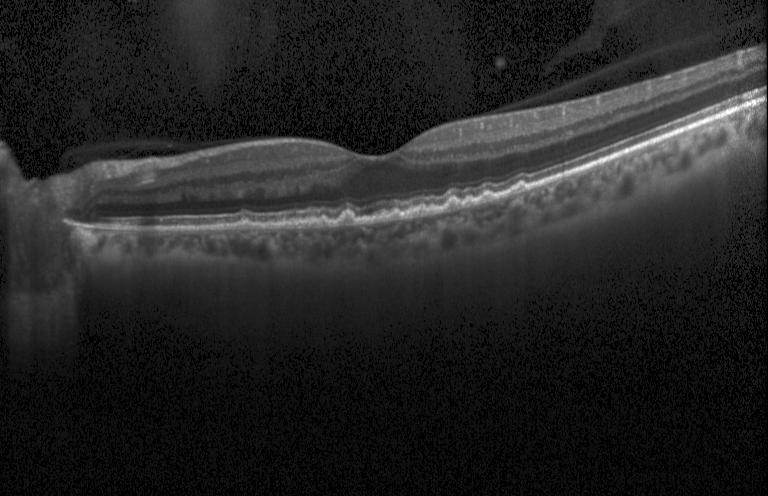
Heidelberg Spectralis · macular scan · spectral-domain OCT · OCT line scan. Impression: multiple drusen.